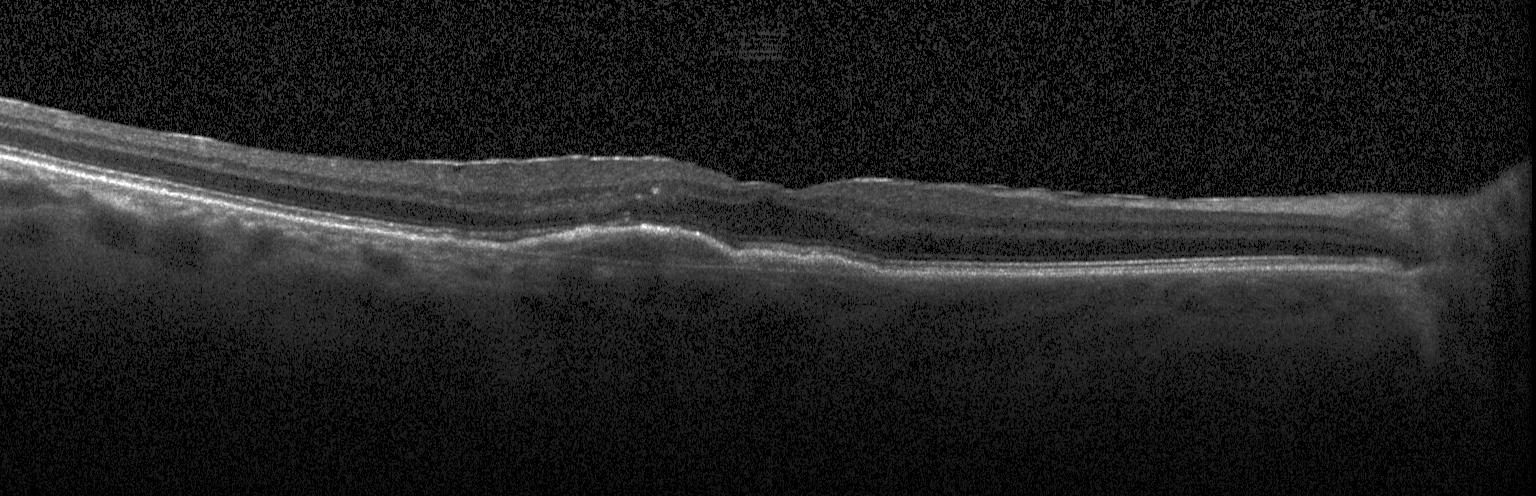 Fovea-centered. Optical coherence tomography B-scan. SD-OCT.
Diagnosis: a choroidal neovascular membrane.